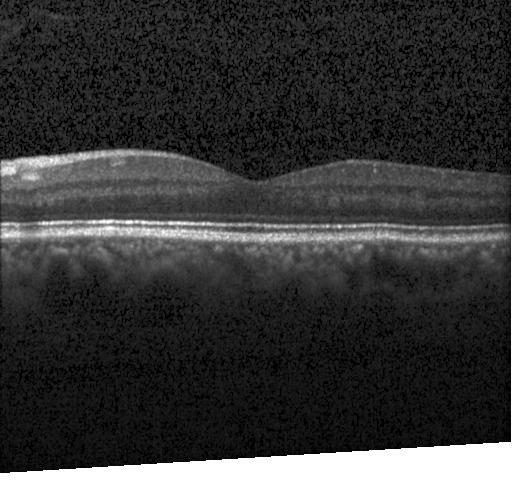
The scan shows no choroidal neovascularization, no diabetic macular edema, and no drusen.